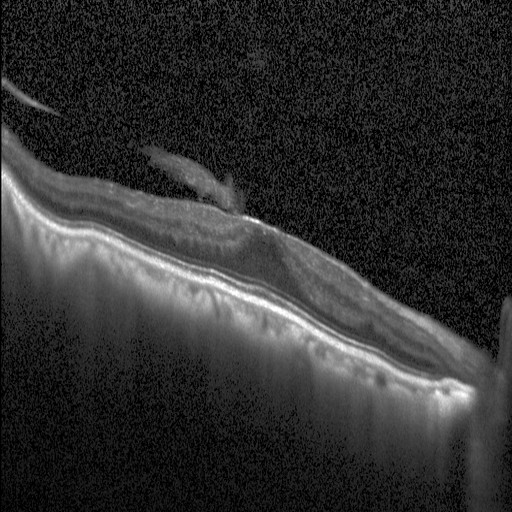

OCT line scan. Macular OCT: diabetic macular edema.